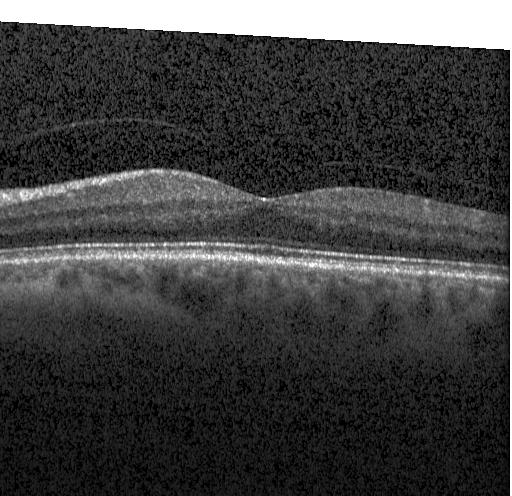

Optical coherence tomography scan; Heidelberg Spectralis OCT system; spectral-domain OCT; centered on the fovea — The scan shows no choroidal neovascularization, no diabetic macular edema, and no drusen.